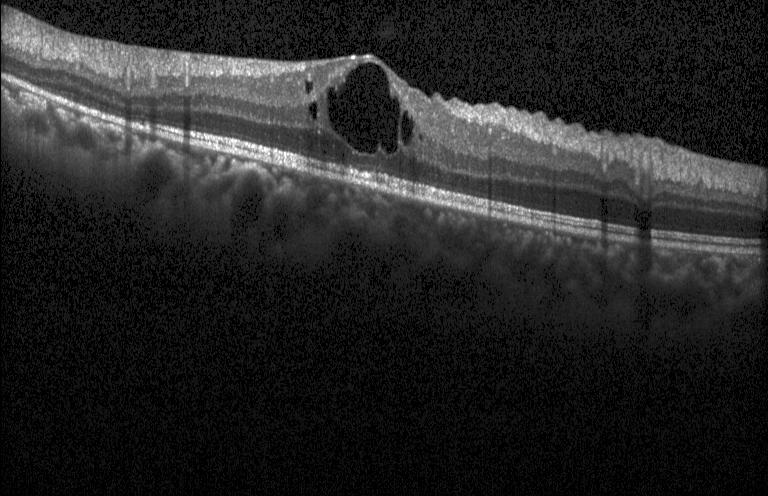 Optical coherence tomography B-scan, Heidelberg Spectralis OCT system — OCT finding: diabetic macular edema (DME).